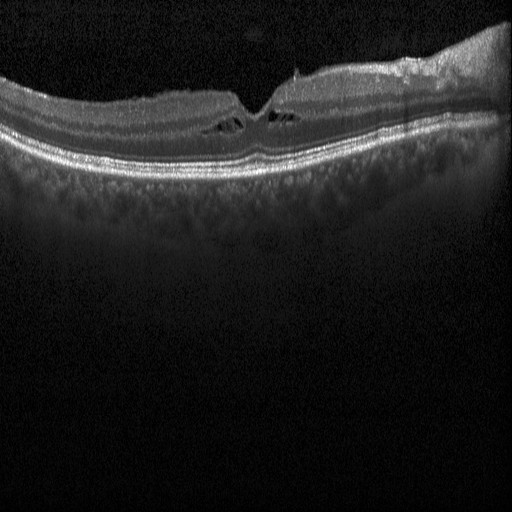
The scan shows diabetic macular edema.